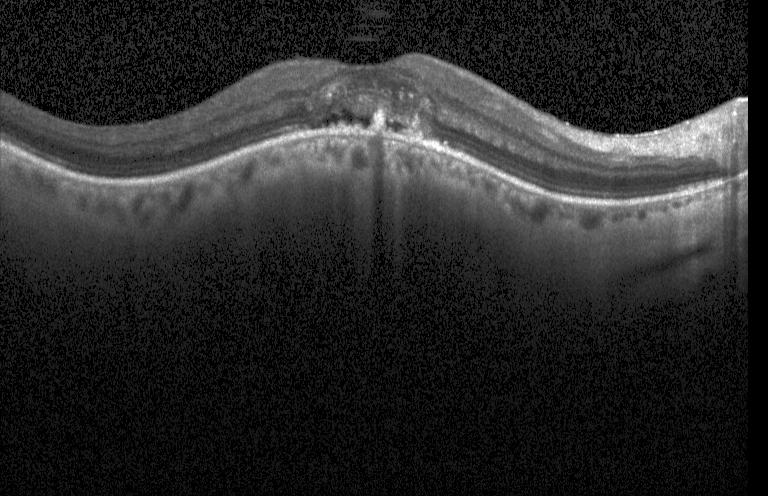

Through the macula · instrument: Heidelberg Spectralis · OCT line scan
OCT finding: a choroidal neovascular membrane.